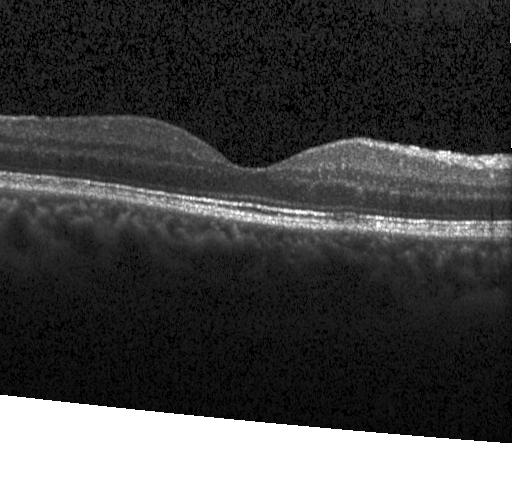

Instrument: Heidelberg Spectralis · spectral-domain optical coherence tomography · OCT B-scan · centered on the fovea — Finding: no evidence of choroidal neovascularization, diabetic macular edema, or drusen.